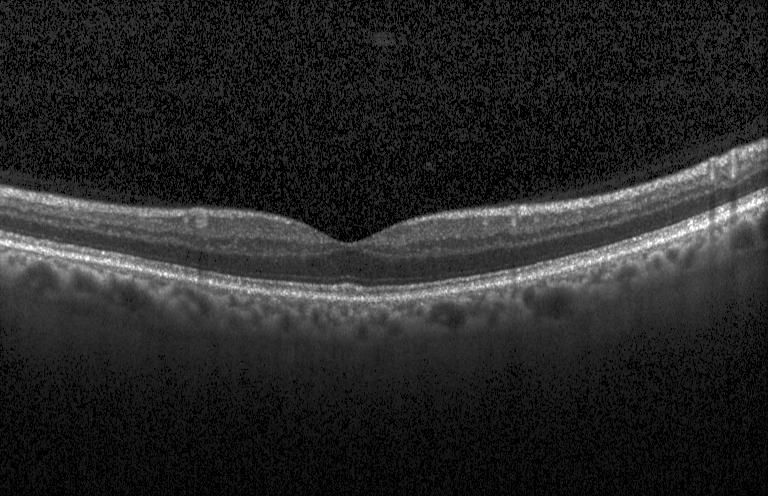

Instrument: Heidelberg Spectralis. Horizontal scan through the fovea. Retinal OCT cross-section. Spectral-domain OCT — Impression: no choroidal neovascularization, no diabetic macular edema, and no drusen.